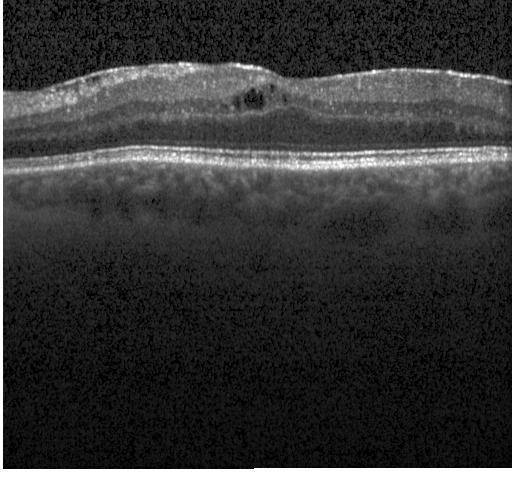

Heidelberg Spectralis OCT system; retinal OCT cross-section; horizontal scan through the fovea.
Diagnosis: diabetic macular edema (DME).